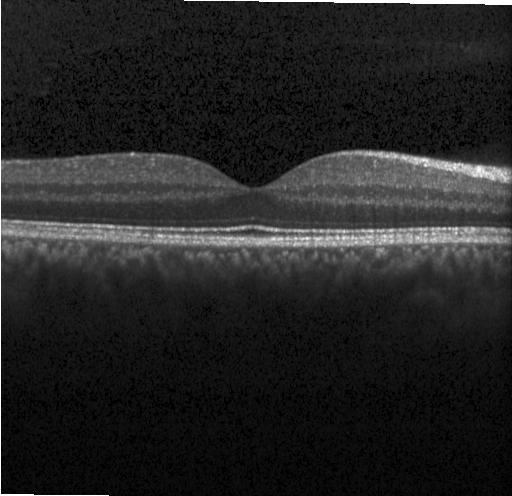 Impression: no evidence of CNV, DME, or drusen.